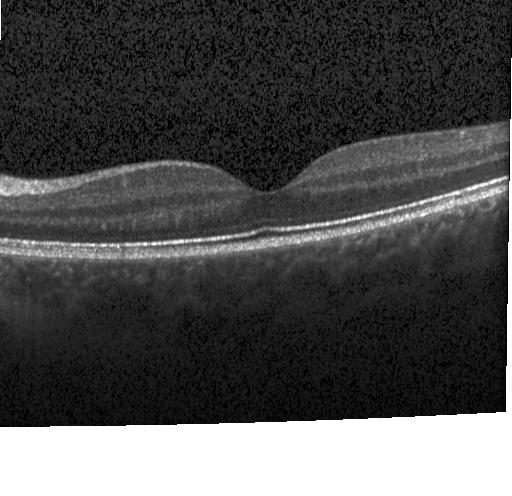 OCT B-scan showing no choroidal neovascularization, no diabetic macular edema, and no drusen.